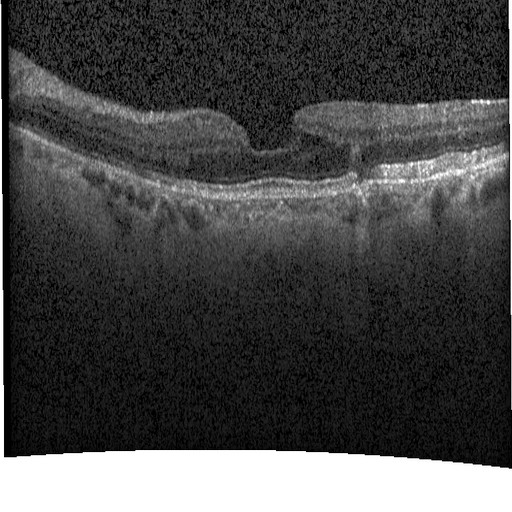

Impression: diabetic macular edema (DME).